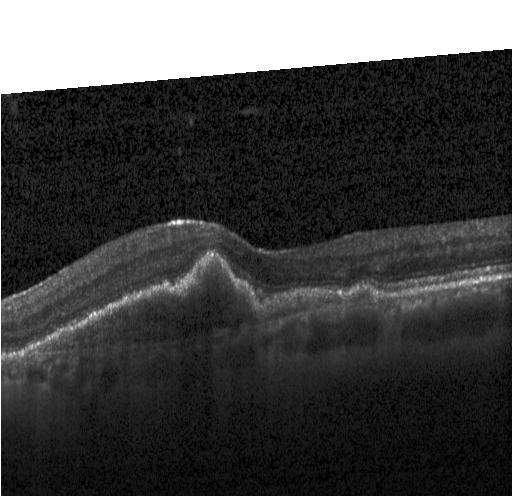

Retinal OCT B-scan — Impression: choroidal neovascularization.